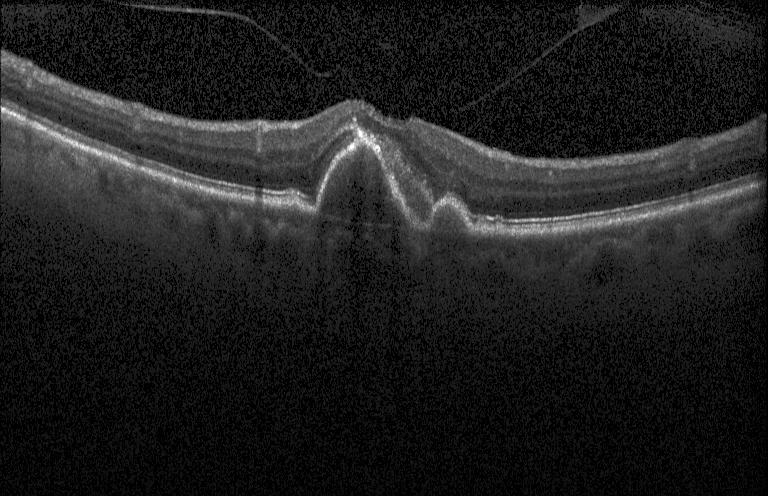

Optical coherence tomography scan
Impression: a choroidal neovascular membrane.